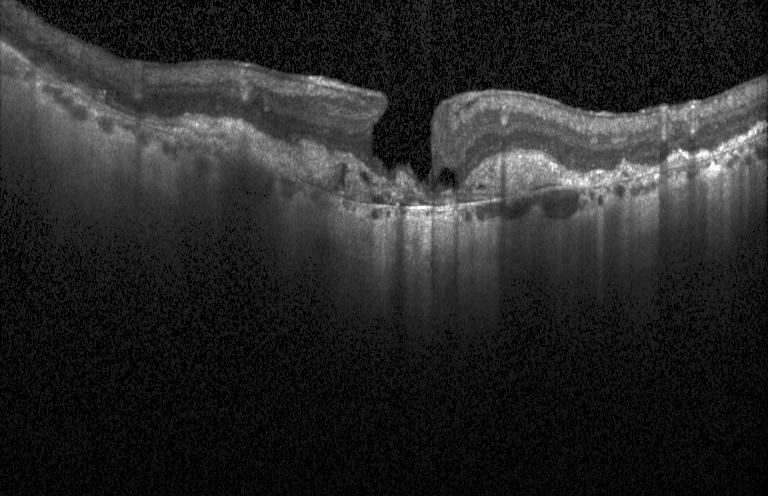
OCT finding: a choroidal neovascular membrane.